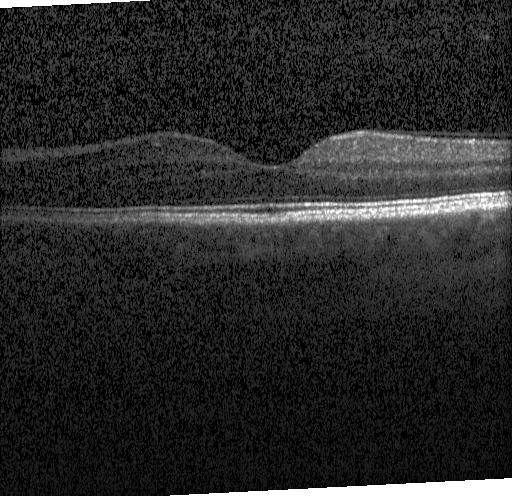

Finding: no evidence of CNV, DME, or drusen.